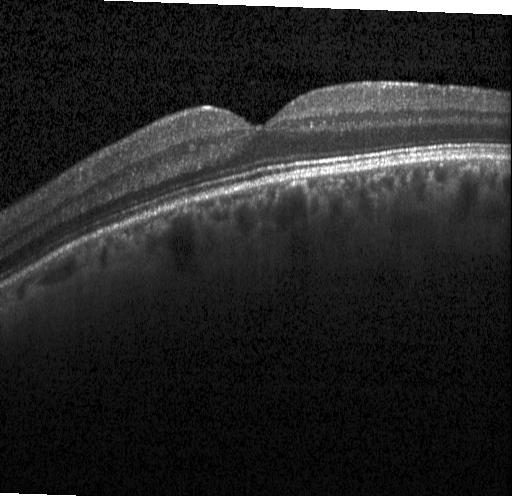
This B-scan demonstrates no evidence of CNV, DME, or drusen.